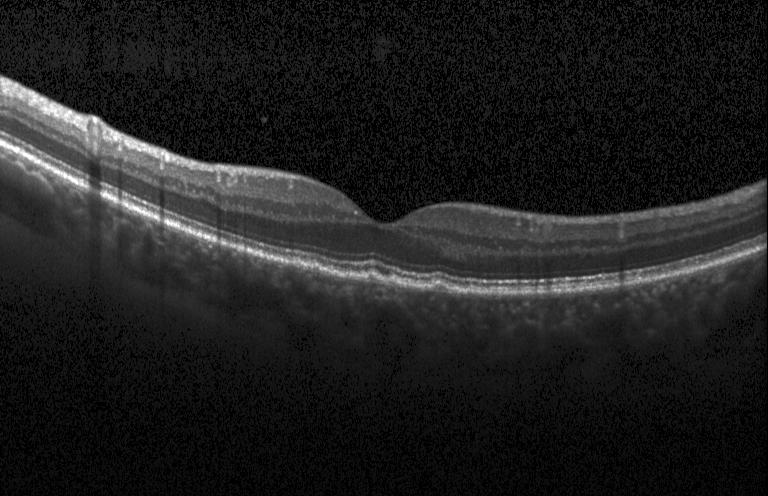

Diagnosis: multiple drusen.